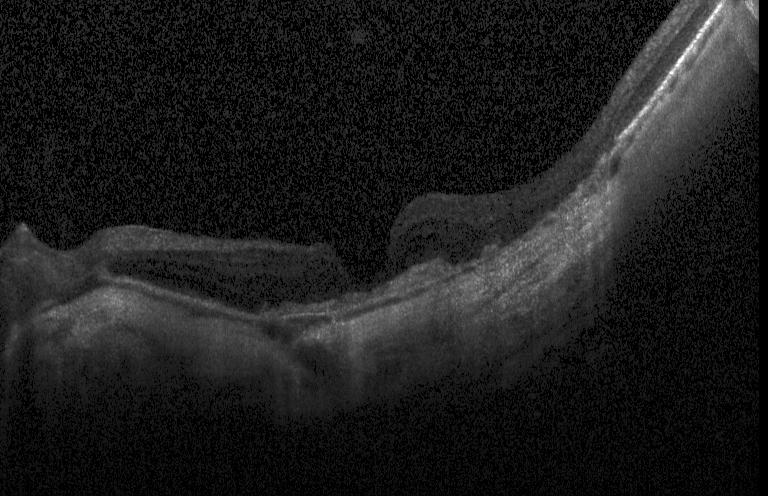

Optical coherence tomography scan — A choroidal neovascular membrane.